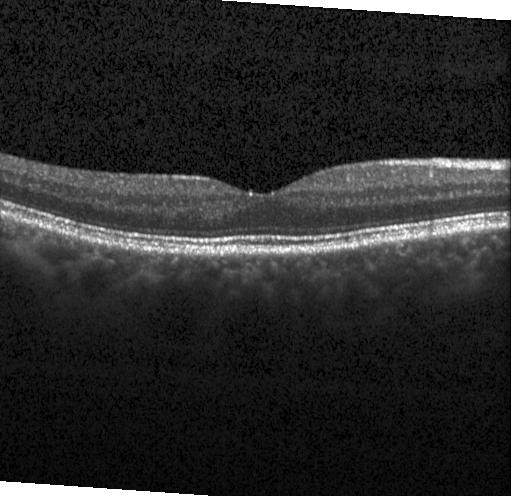 Macular OCT: no choroidal neovascularization, no diabetic macular edema, and no drusen.